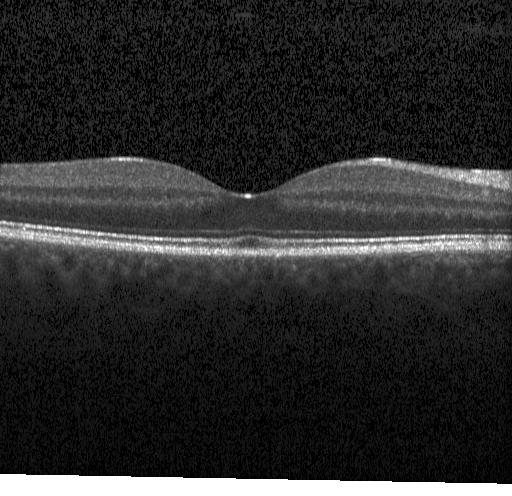
Heidelberg Spectralis. Retinal OCT cross-section — Assessment: neither choroidal neovascularization, diabetic macular edema, nor drusen.